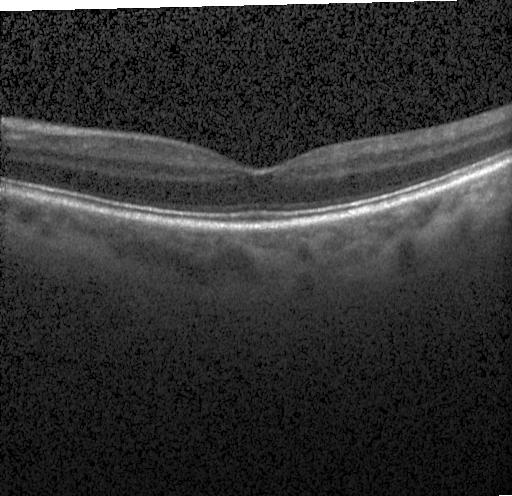 Macular OCT: no choroidal neovascularization, no diabetic macular edema, and no drusen.